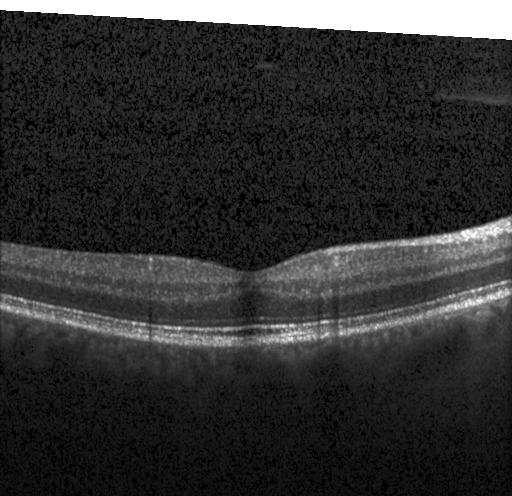
Retinal OCT cross-section · through the macula. Dx: no evidence of choroidal neovascularization, diabetic macular edema, or drusen.